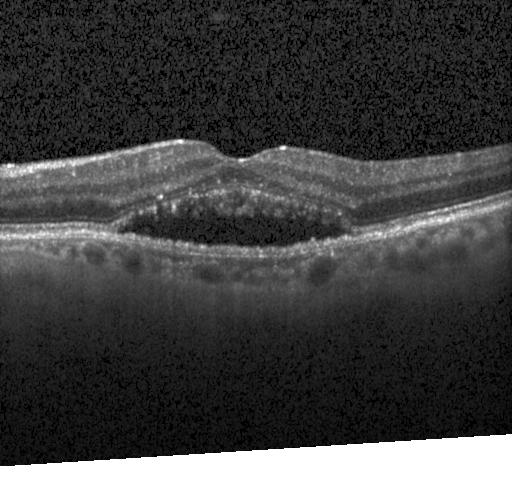
Retinal OCT cross-section showing a choroidal neovascular membrane.